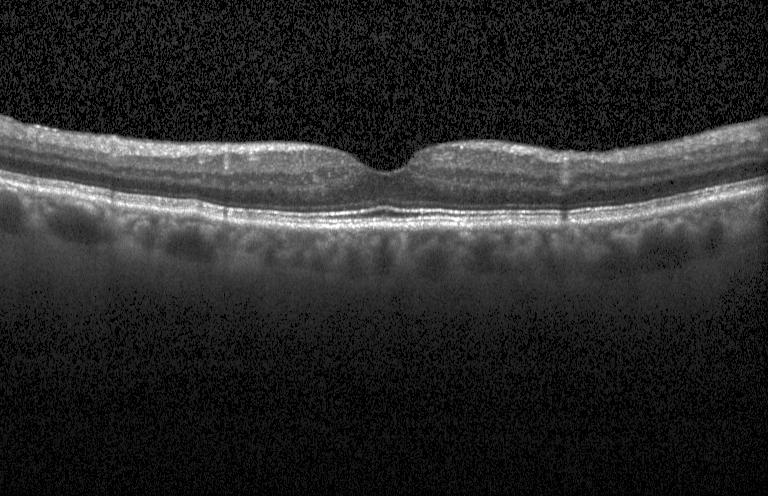 Retinal OCT B-scan
Dx: no choroidal neovascularization, no diabetic macular edema, and no drusen.